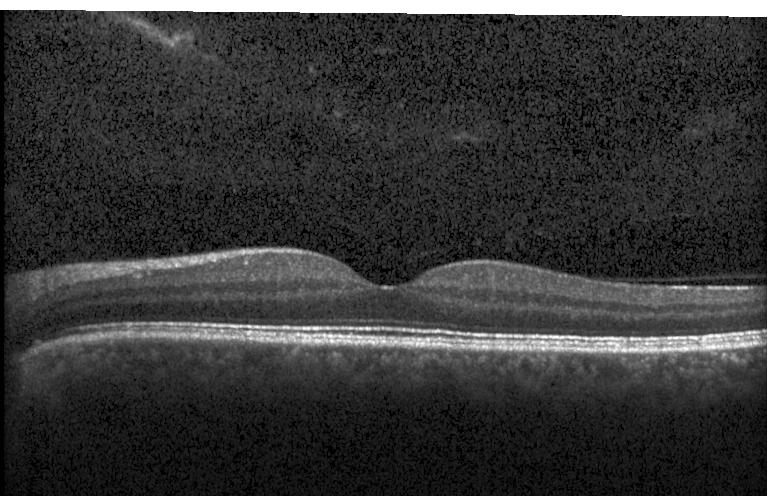 SD-OCT, macular scan, acquired on a Heidelberg Spectralis, retinal OCT cross-section — Diagnosis: no choroidal neovascularization, diabetic macular edema, or drusen.